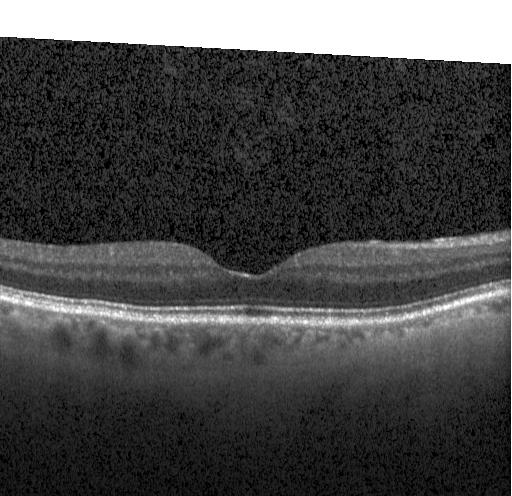
Optical coherence tomography B-scan. Finding: no evidence of CNV, DME, or drusen.